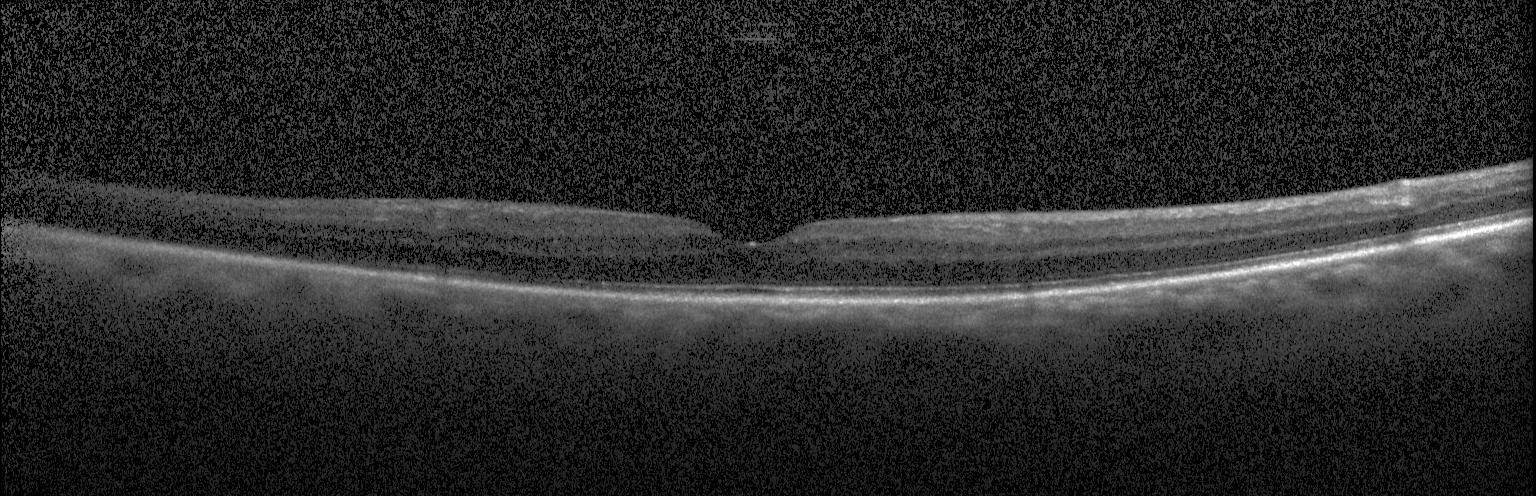
OCT B-scan
This B-scan demonstrates no choroidal neovascularization, no diabetic macular edema, and no drusen.